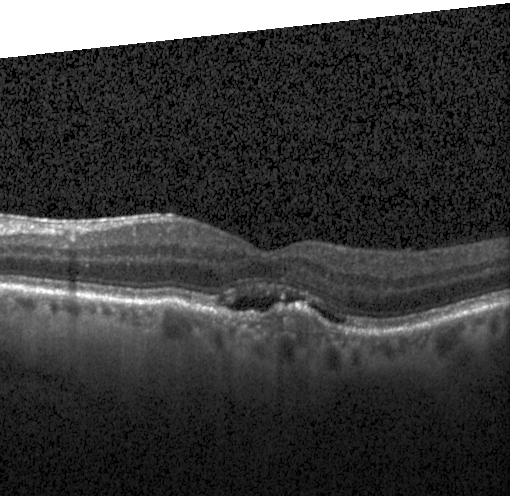

Diagnosis: a choroidal neovascular membrane.